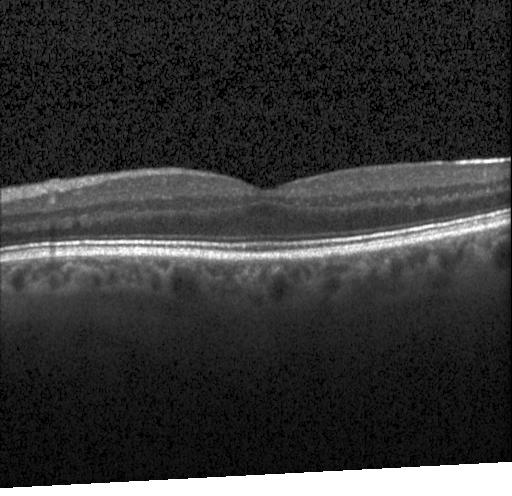

Retinal OCT cross-section · acquired on a Heidelberg Spectralis
Diagnosis: no CNV, no DME, and no drusen.